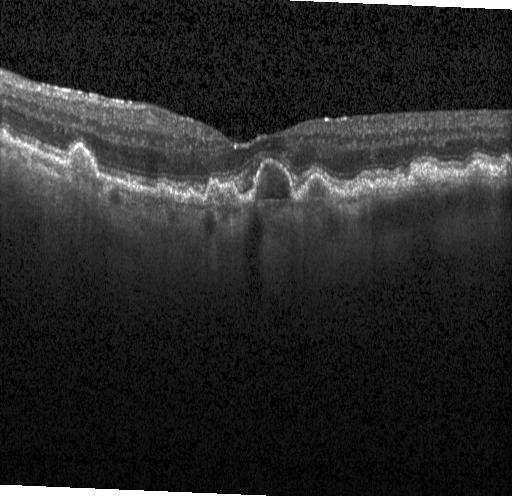

Retinal OCT cross-section; fovea-centered; Heidelberg Spectralis
OCT finding: drusen.